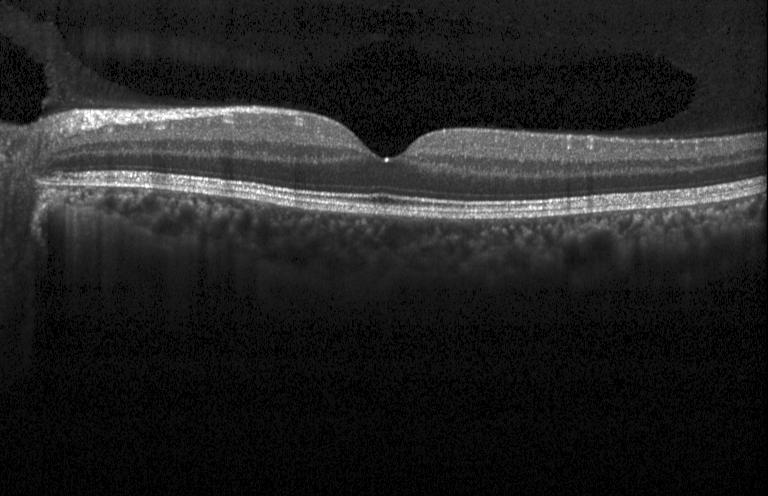
Spectral-domain optical coherence tomography. OCT line scan. Through the macula. Finding: no CNV, DME, or drusen.